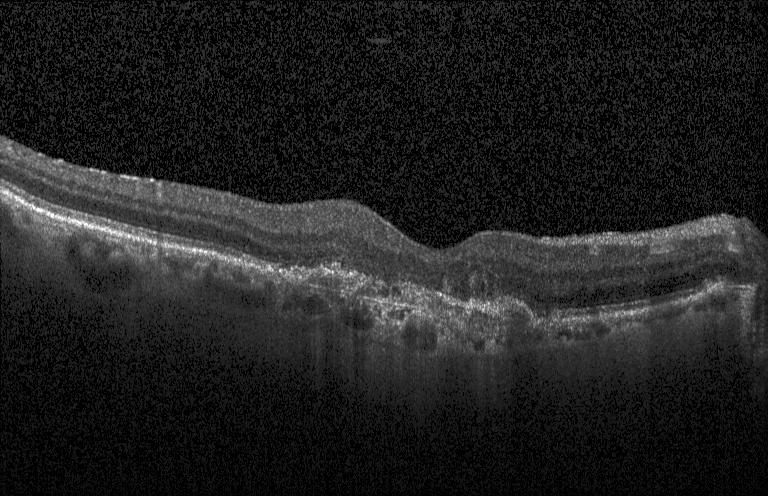

Retinal OCT B-scan.
This B-scan demonstrates choroidal neovascularization.